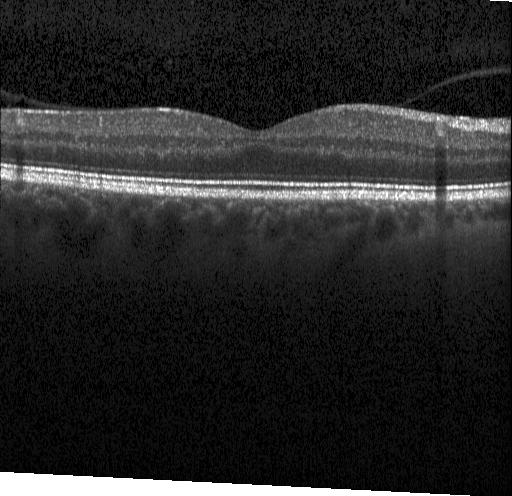
Optical coherence tomography scan — No evidence of choroidal neovascularization, diabetic macular edema, or drusen.